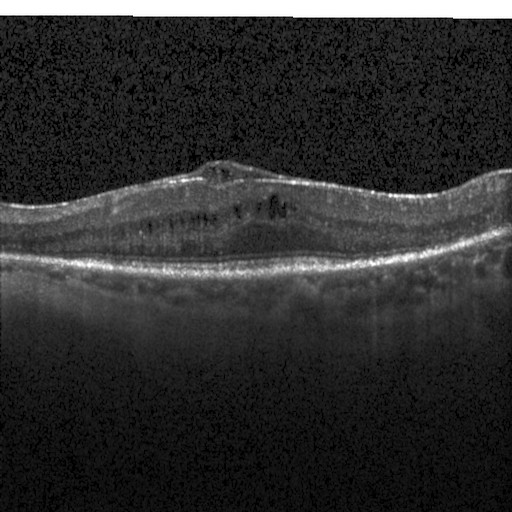
Spectral-domain OCT B-scan: DME.